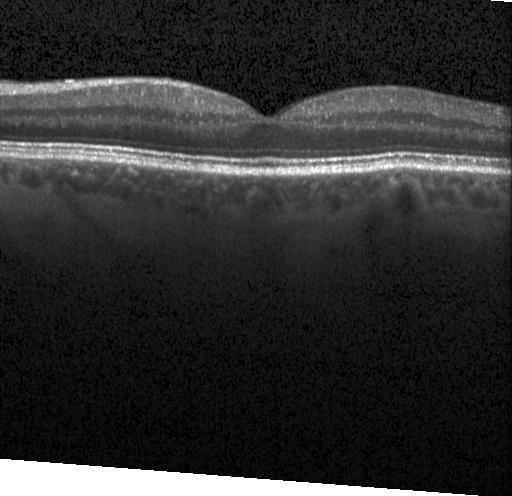 Optical coherence tomography B-scan, spectral-domain optical coherence tomography, macular scan.
Dx: no choroidal neovascularization, diabetic macular edema, or drusen.